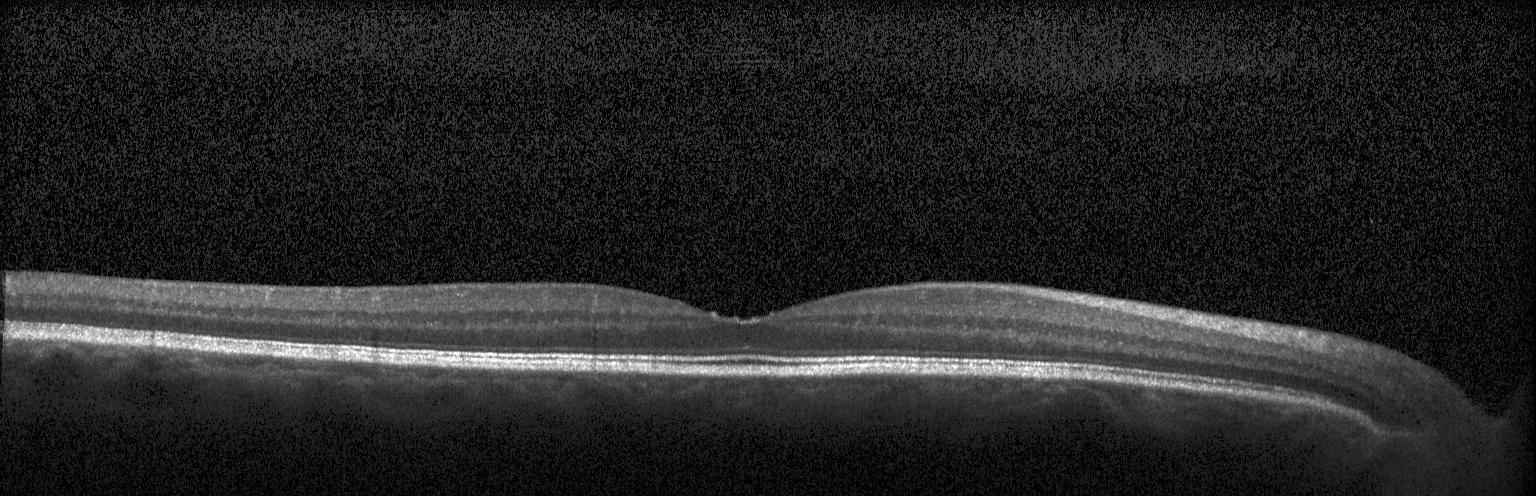 Horizontal scan through the fovea, Heidelberg Spectralis OCT system, spectral-domain OCT, optical coherence tomography B-scan.
Diagnosis: no evidence of CNV, DME, or drusen.